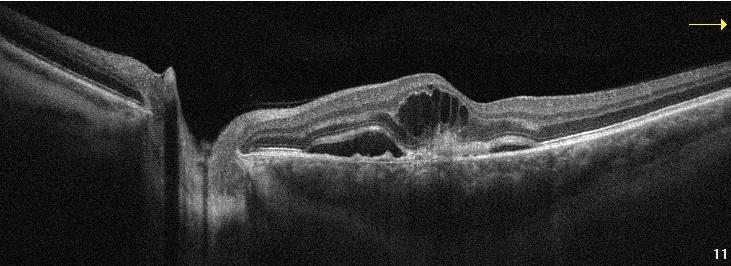
Macular OCT: AMD.